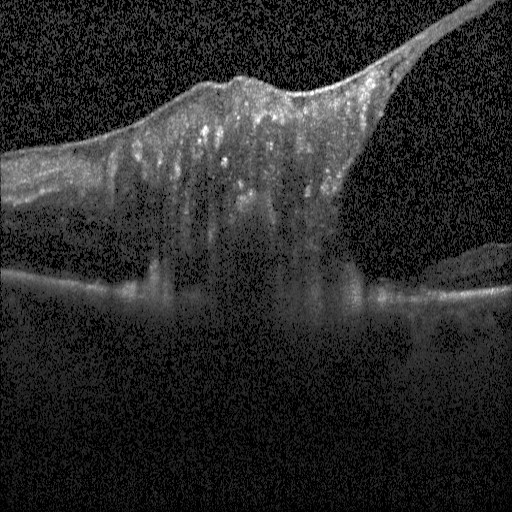

OCT scan showing diabetic macular edema (DME).